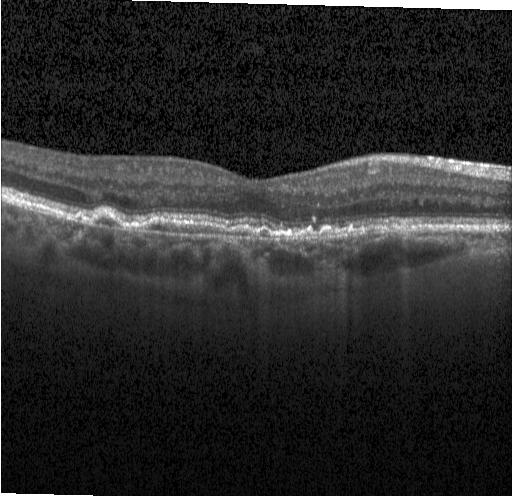 Retinal OCT cross-section — Macular OCT: a choroidal neovascular membrane.